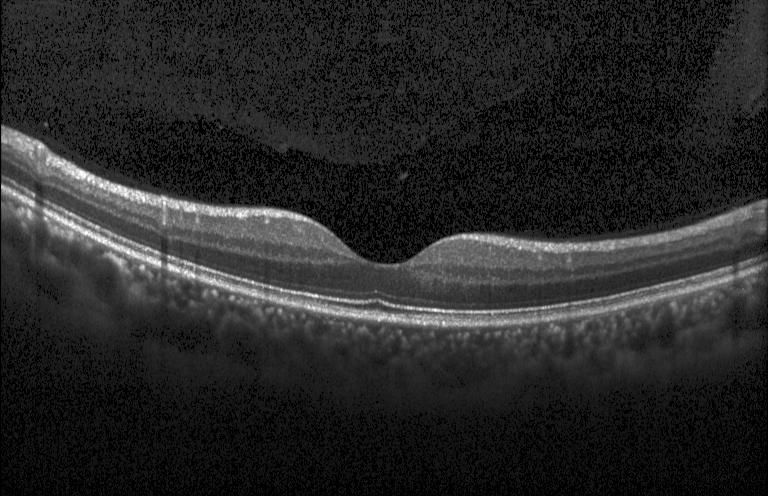 Impression: neither CNV, DME, nor drusen.